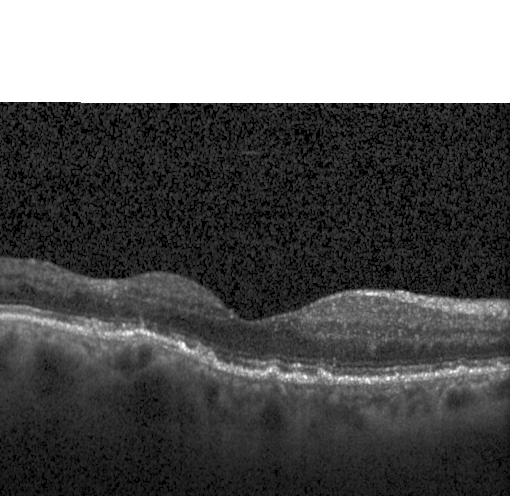

Retinal OCT cross-section — Drusen.